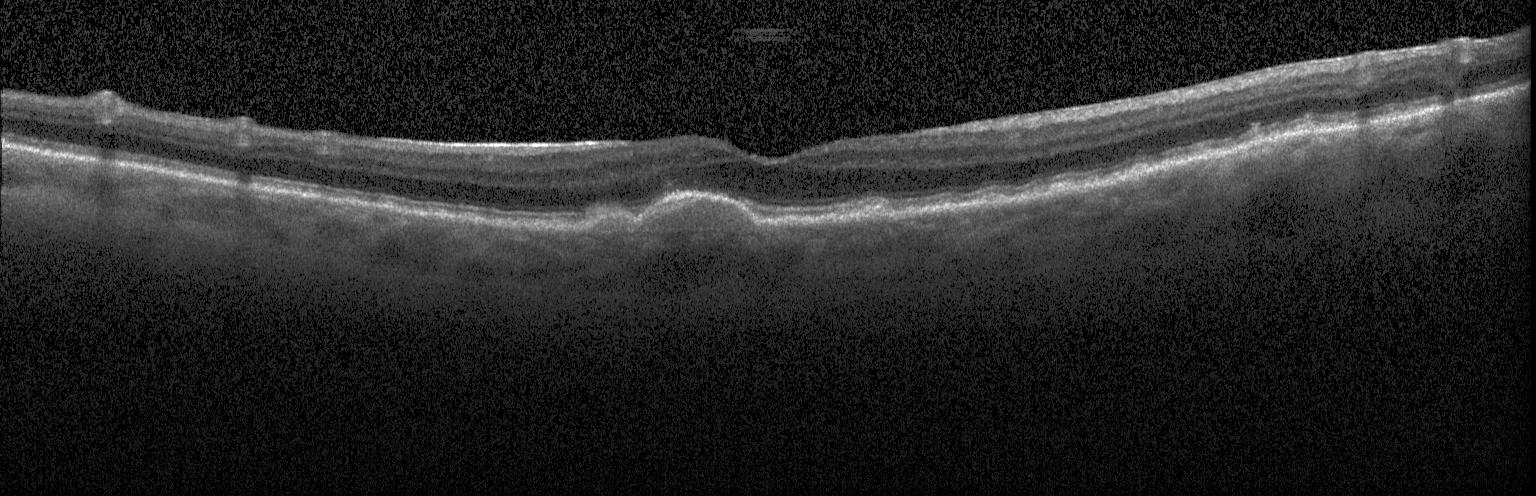

OCT line scan, Heidelberg Spectralis, fovea-centered.
The scan shows drusen.